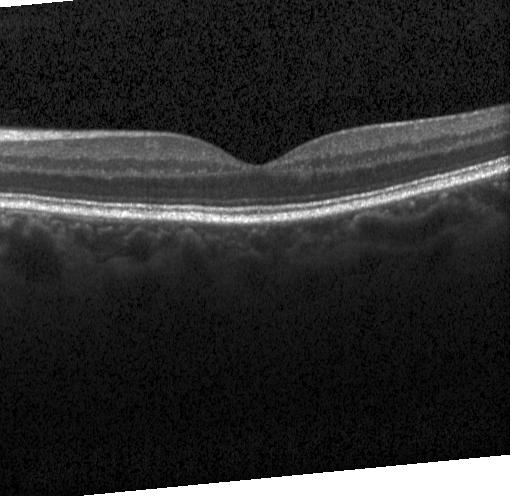

Impression: no choroidal neovascularization, diabetic macular edema, or drusen.